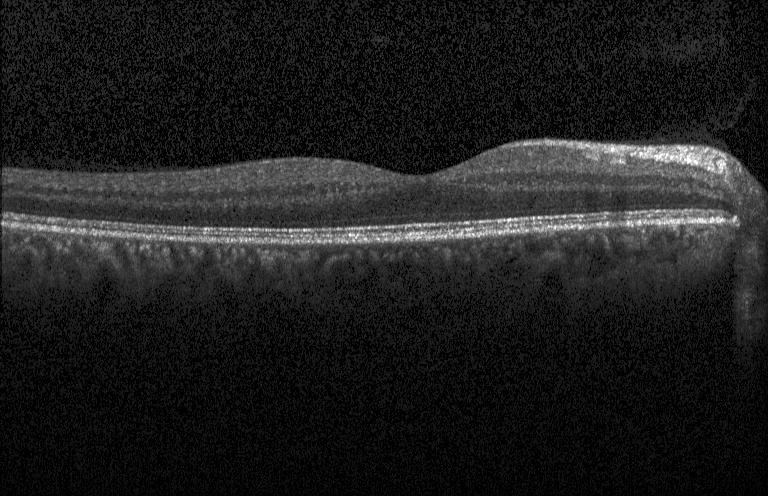
Retinal OCT B-scan. Centered on the fovea
Finding: neither choroidal neovascularization, diabetic macular edema, nor drusen.